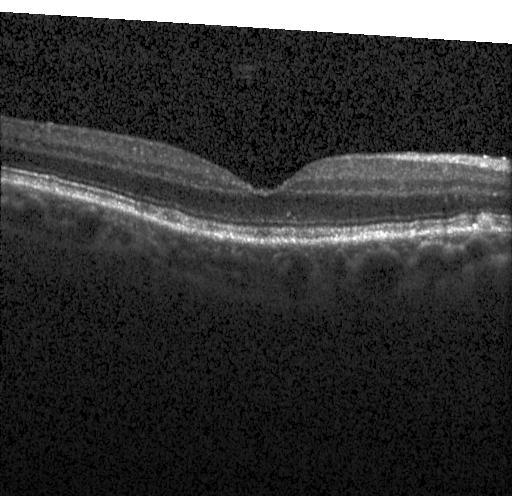 OCT B-scan; acquired on a Heidelberg Spectralis. Finding: multiple drusen.